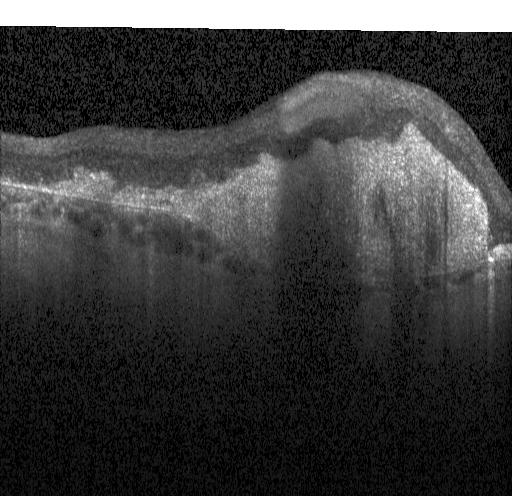

Macular OCT: a choroidal neovascular membrane.